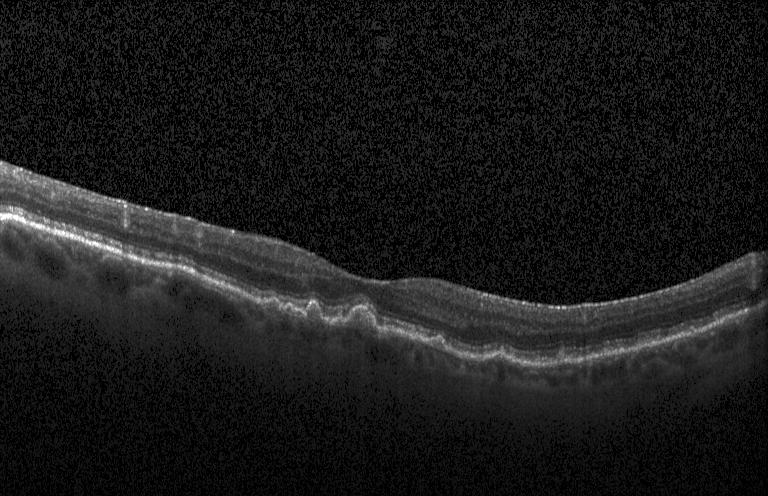
OCT finding: sub-RPE drusenoid deposits.